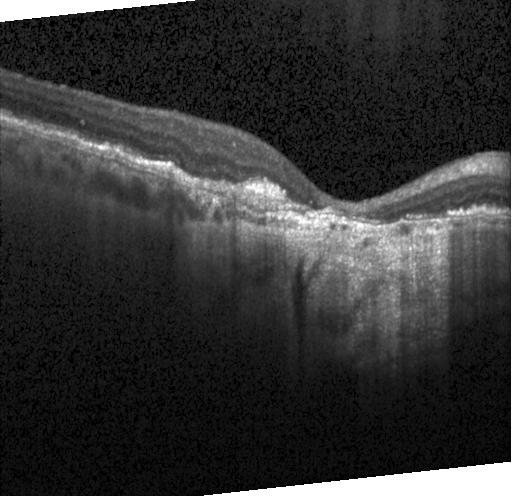

Retinal OCT cross-section
A choroidal neovascular membrane.